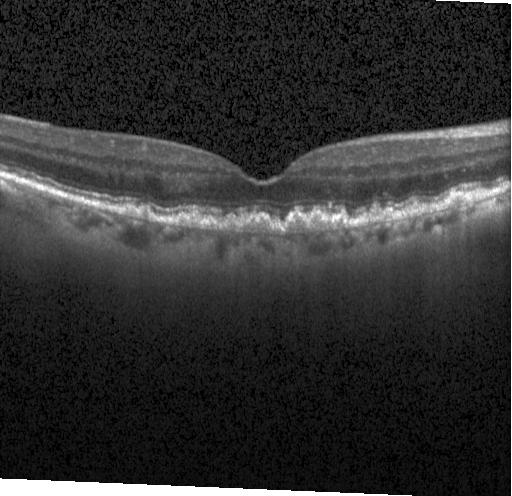
Spectral-domain optical coherence tomography, macular scan, optical coherence tomography B-scan
Assessment: drusen.